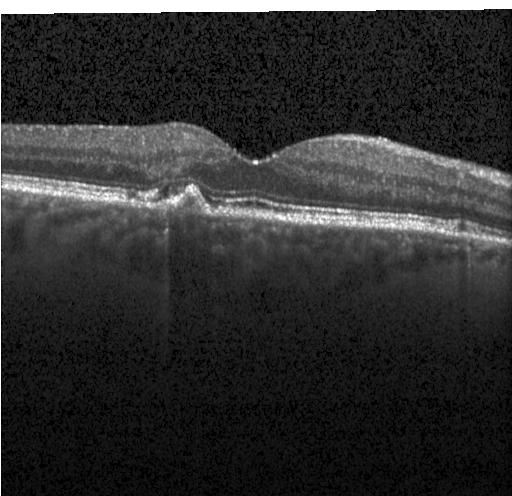
Impression: multiple drusen.